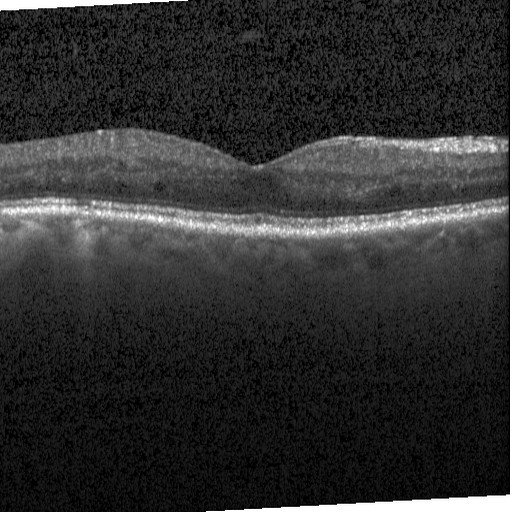 OCT finding: diabetic macular edema.